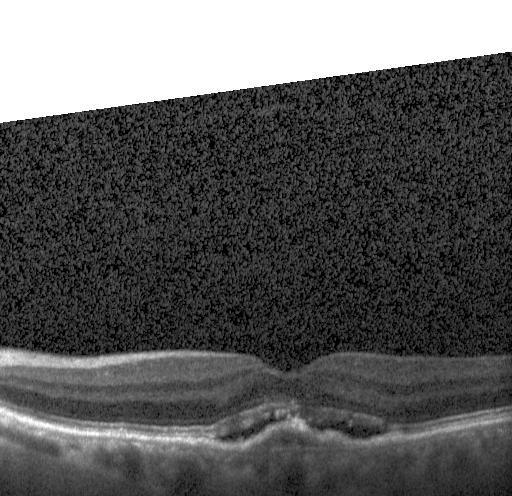
OCT line scan. Heidelberg Spectralis OCT system — Assessment: a choroidal neovascular membrane.